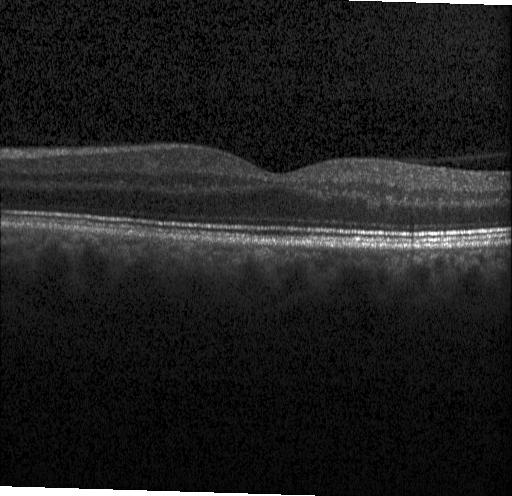
Retinal OCT cross-section.
Finding: no choroidal neovascularization, no diabetic macular edema, and no drusen.